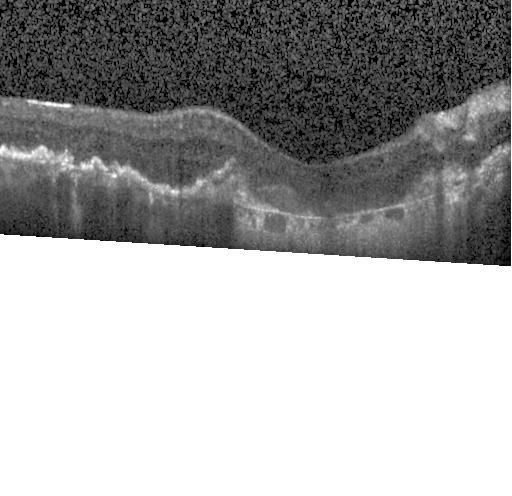

Fovea-centered; spectral-domain optical coherence tomography; instrument: Heidelberg Spectralis; optical coherence tomography scan
Macular OCT: CNV.